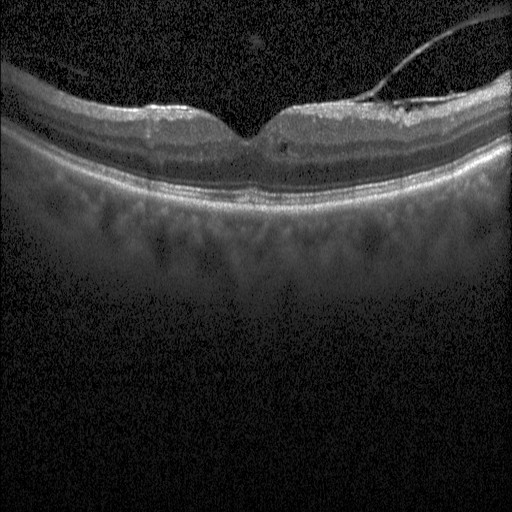

The scan shows diabetic macular edema (DME).